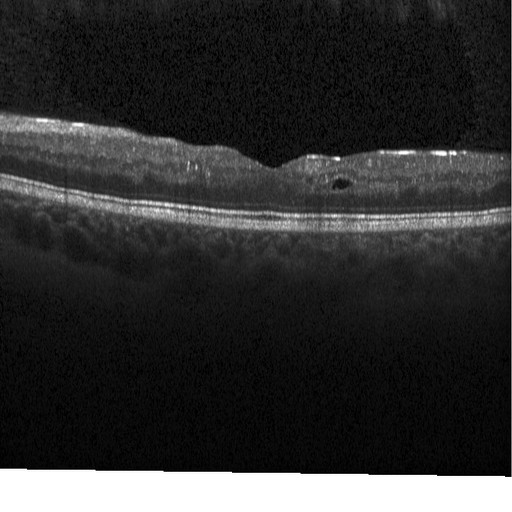

Spectral-domain OCT, instrument: Heidelberg Spectralis, OCT B-scan, horizontal scan through the fovea.
OCT finding: DME.